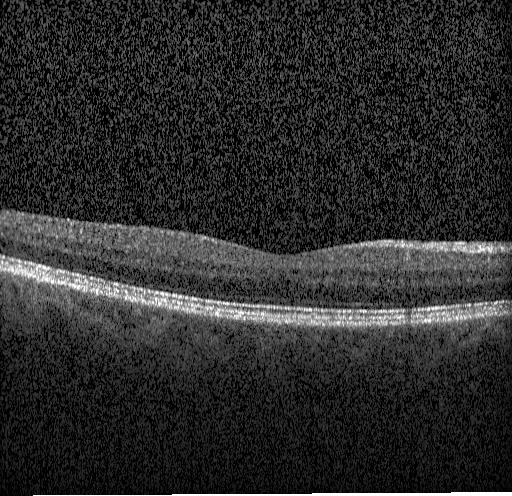

OCT B-scan. The scan shows neither choroidal neovascularization, diabetic macular edema, nor drusen.